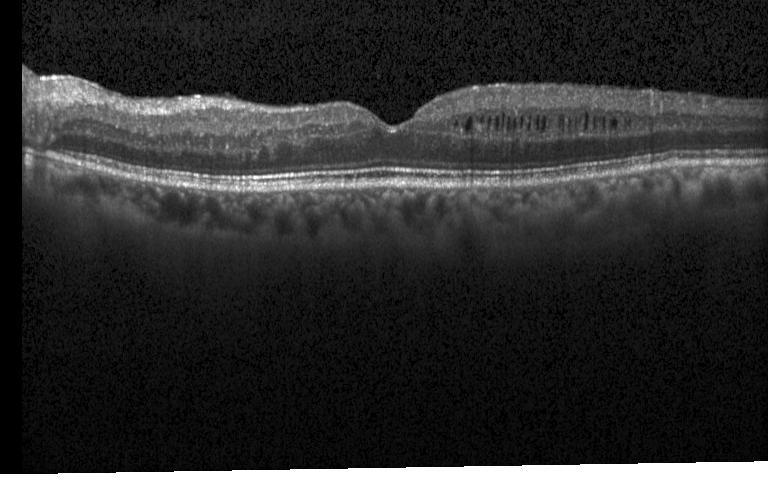
Retinal OCT B-scan — The scan shows DME.